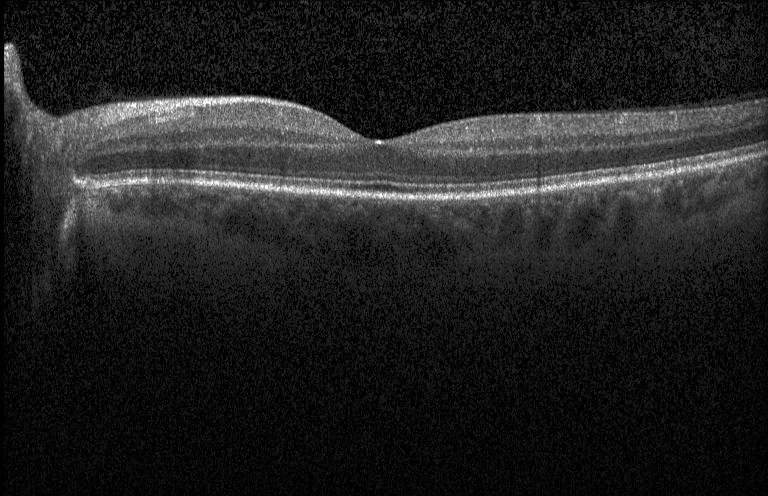

Spectral-domain OCT, optical coherence tomography scan, instrument: Heidelberg Spectralis, centered on the fovea. Impression: neither choroidal neovascularization, diabetic macular edema, nor drusen.